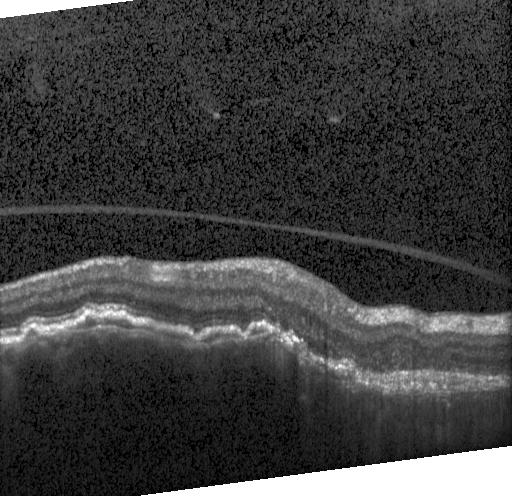
SD-OCT · instrument: Heidelberg Spectralis · fovea-centered · optical coherence tomography B-scan. Finding: choroidal neovascularization.